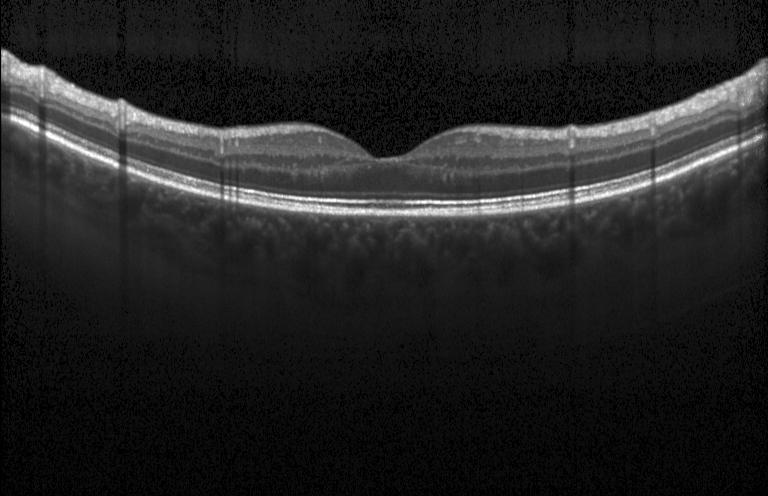

OCT B-scan. Heidelberg Spectralis OCT system.
No CNV, DME, or drusen.